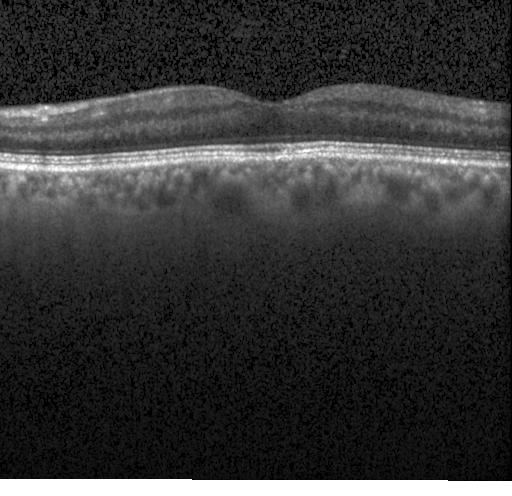

No evidence of CNV, DME, or drusen.